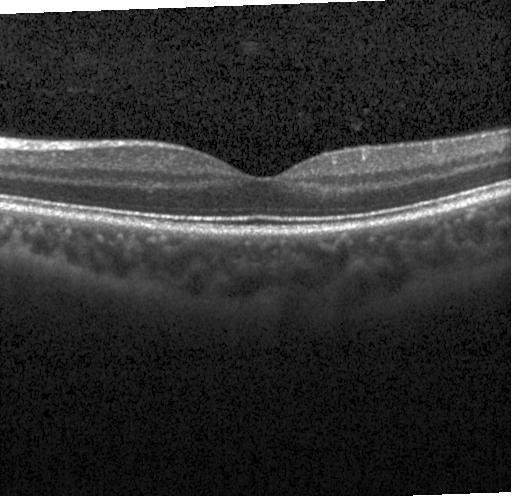
Impression: no evidence of CNV, DME, or drusen.